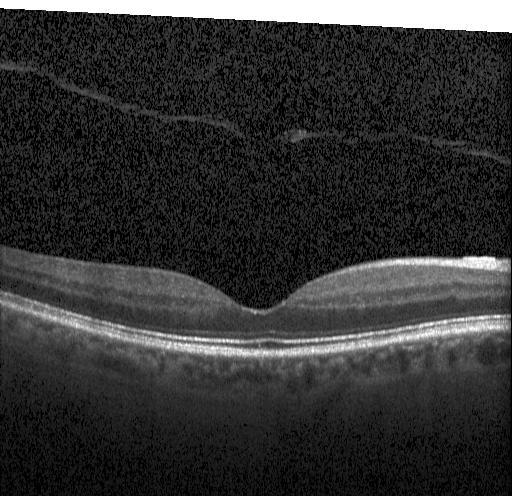 Diagnosis: no choroidal neovascularization, no diabetic macular edema, and no drusen.